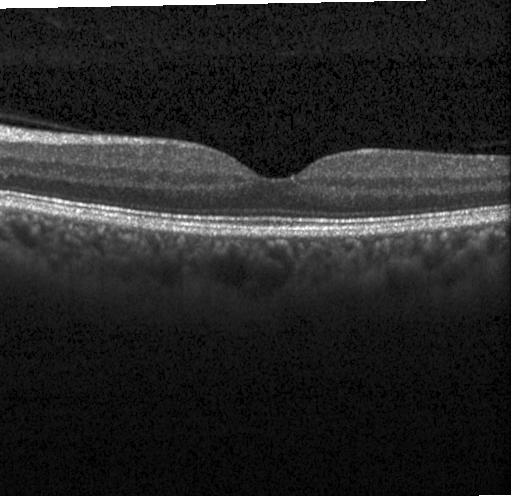

Acquired on a Heidelberg Spectralis. Spectral-domain optical coherence tomography. Optical coherence tomography scan
Macular OCT: no choroidal neovascularization, no diabetic macular edema, and no drusen.